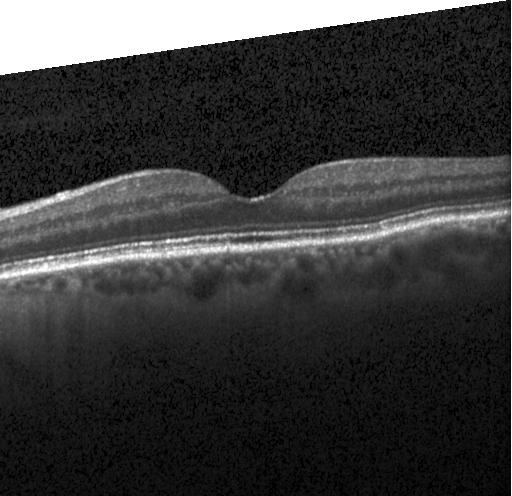
Impression: no choroidal neovascularization, diabetic macular edema, or drusen.